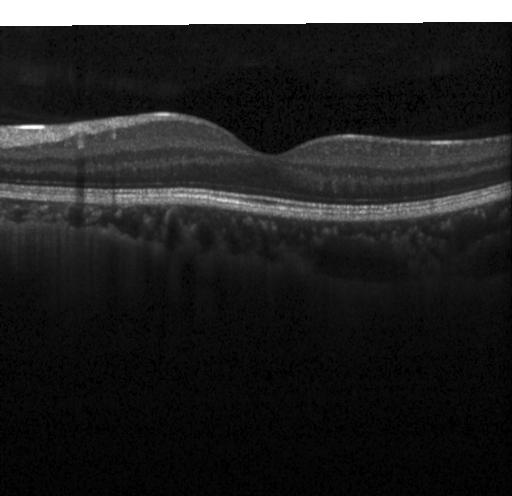 Retinal OCT B-scan; instrument: Heidelberg Spectralis; through the macula — Diagnosis: no choroidal neovascularization, no diabetic macular edema, and no drusen.